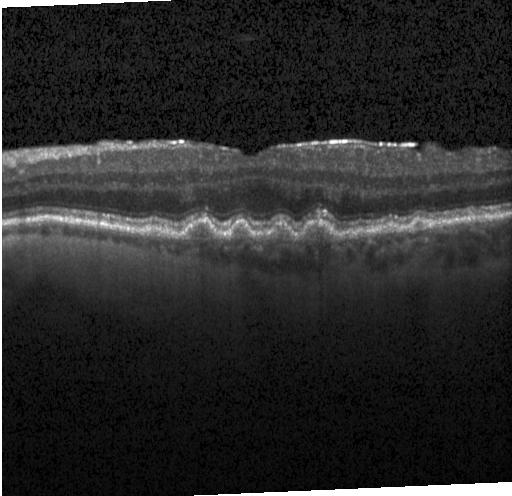 Retinal OCT cross-section showing multiple drusen.